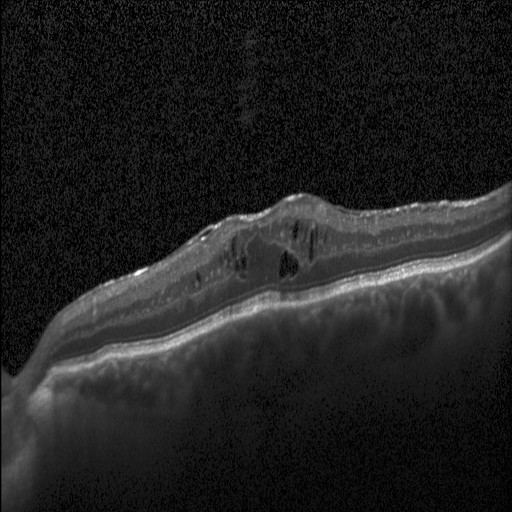 OCT scan showing diabetic macular edema (DME).